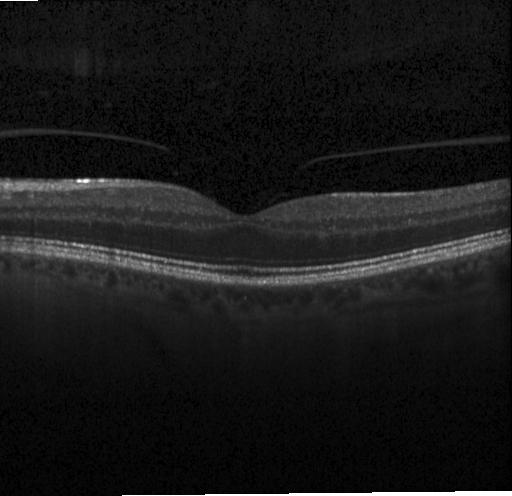
Optical coherence tomography scan; Heidelberg Spectralis; spectral-domain OCT; macular scan.
This B-scan demonstrates no choroidal neovascularization, no diabetic macular edema, and no drusen.